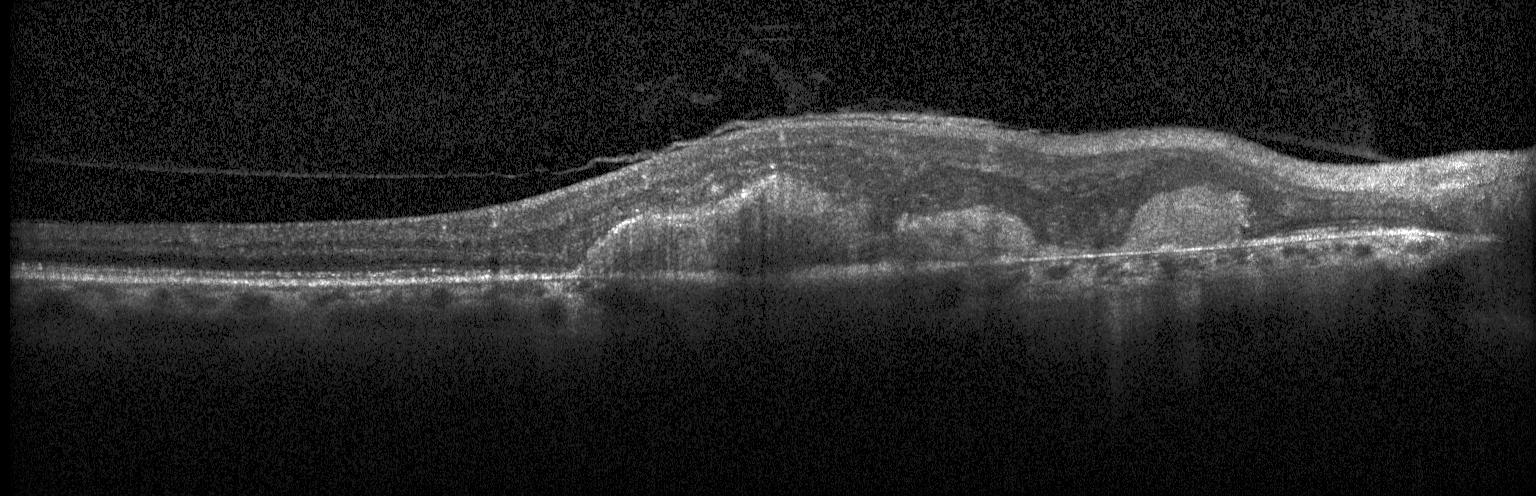

Heidelberg Spectralis OCT system; OCT B-scan — This B-scan demonstrates choroidal neovascularization (CNV).